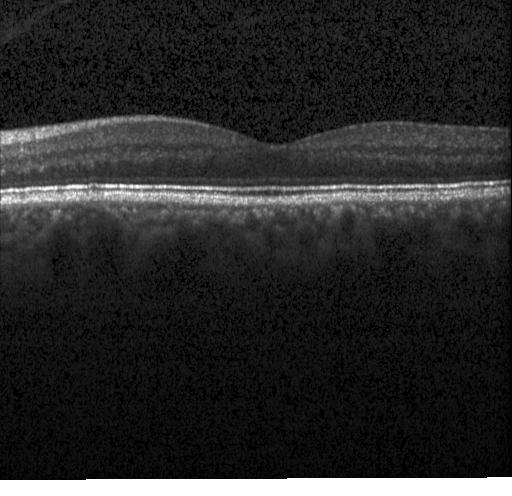 Retinal OCT cross-section; instrument: Heidelberg Spectralis; through the macula. Diagnosis: no CNV, DME, or drusen.